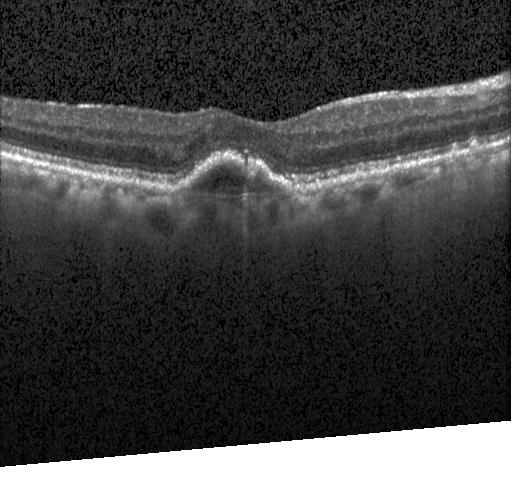

Spectral-domain OCT B-scan: a choroidal neovascular membrane.